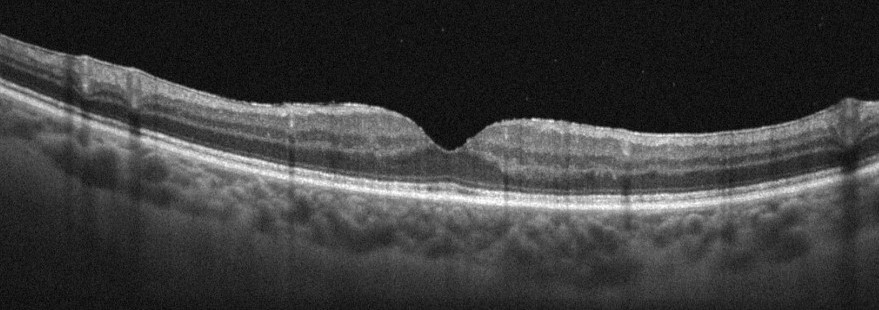 Macular scan, retinal OCT B-scan, Optovue Avanti RTVue XR — Macular OCT: no evidence of AMD, DME, ERM, RAO, RVO, or VID.